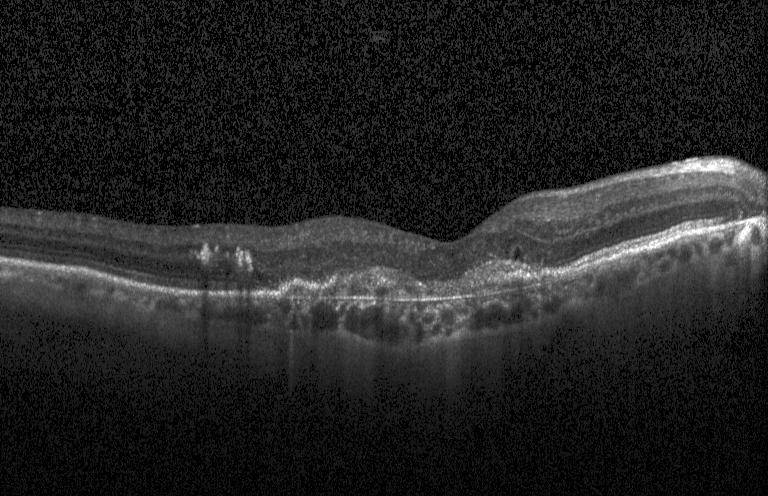

This B-scan demonstrates choroidal neovascularization (CNV).